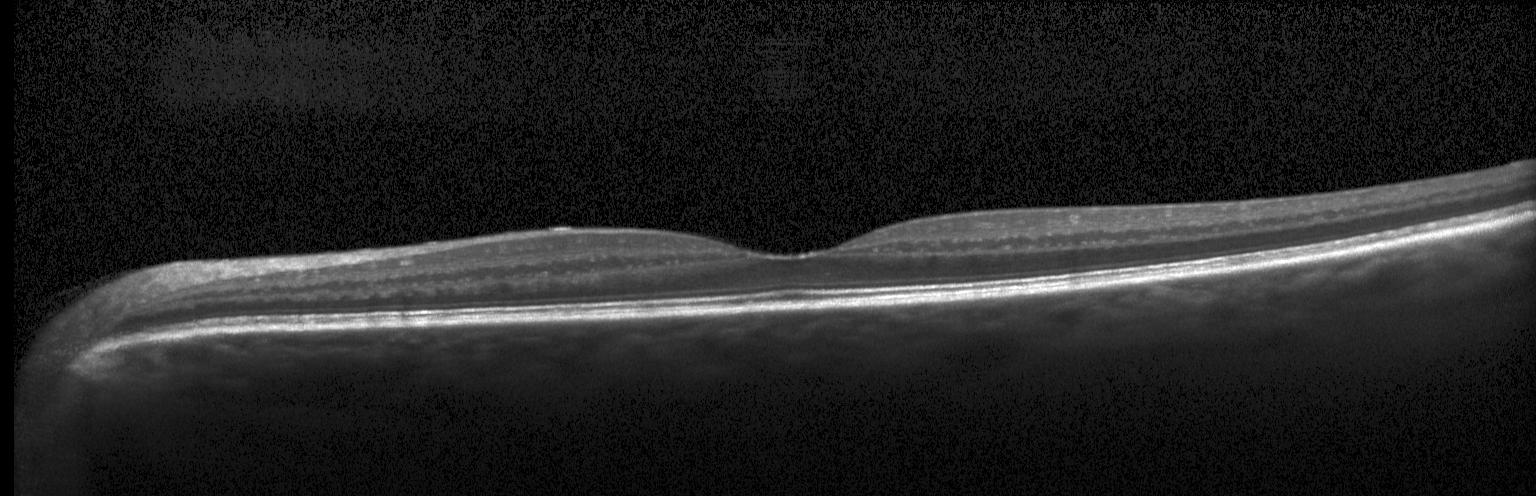
Retinal OCT B-scan · Heidelberg Spectralis · centered on the fovea. This B-scan demonstrates no CNV, no DME, and no drusen.